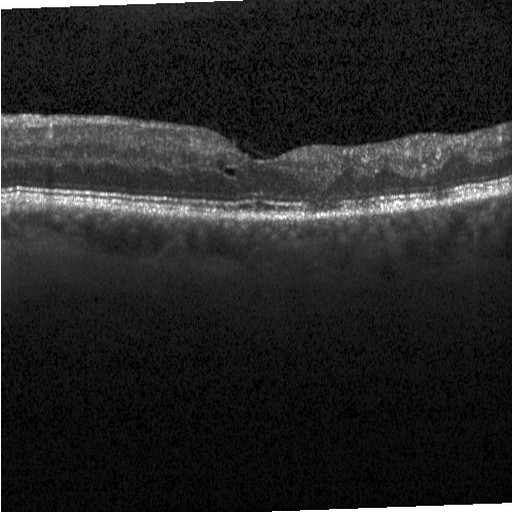

Spectral-domain optical coherence tomography; fovea-centered; retinal OCT cross-section — This B-scan demonstrates diabetic macular edema (DME).